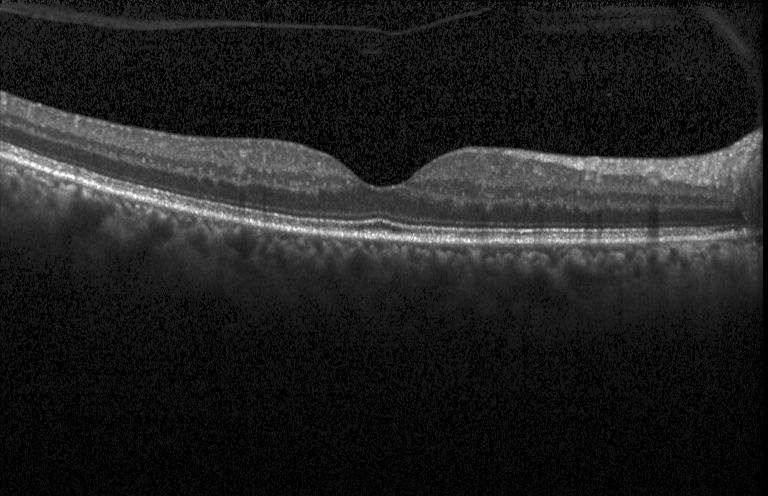 Retinal OCT B-scan; SD-OCT.
Assessment: no CNV, DME, or drusen.